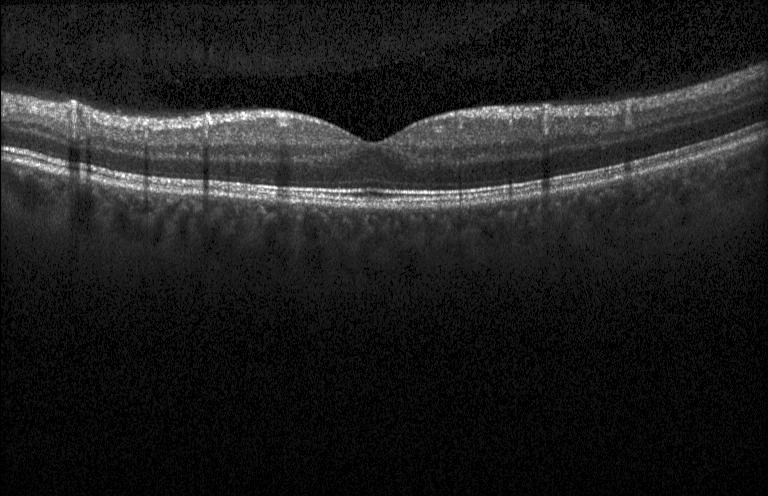
OCT B-scan. Spectral-domain optical coherence tomography. Horizontal scan through the fovea. Acquired on a Heidelberg Spectralis — Dx: no evidence of choroidal neovascularization, diabetic macular edema, or drusen.